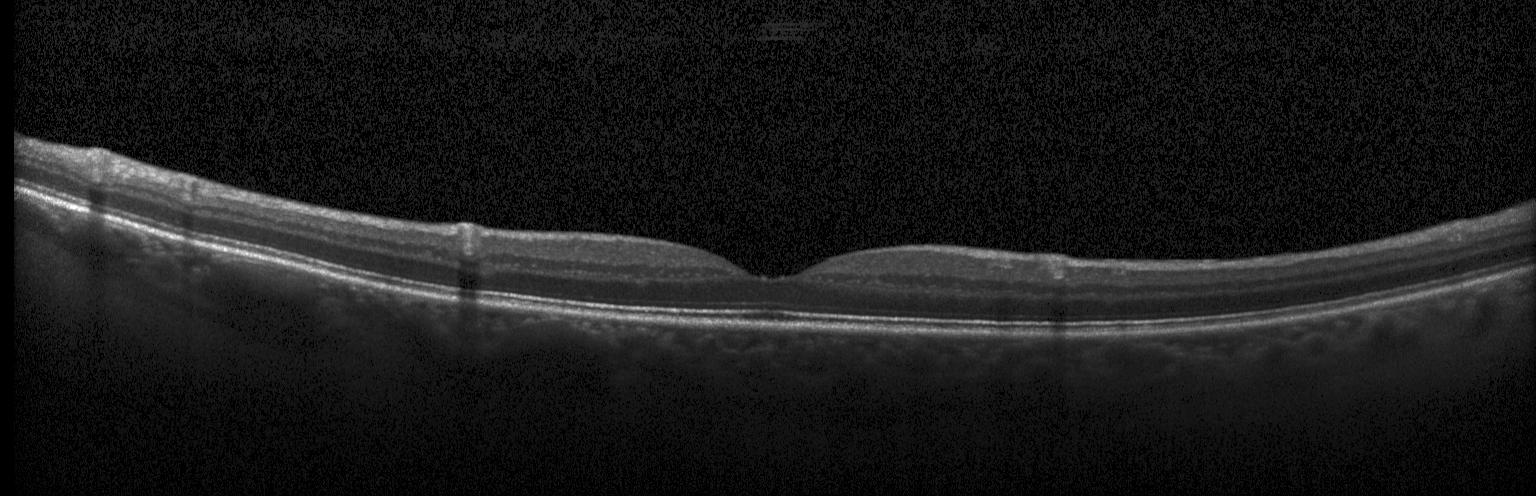 Spectral-domain optical coherence tomography. Heidelberg Spectralis OCT system. OCT B-scan. Fovea-centered — Finding: no evidence of choroidal neovascularization, diabetic macular edema, or drusen.